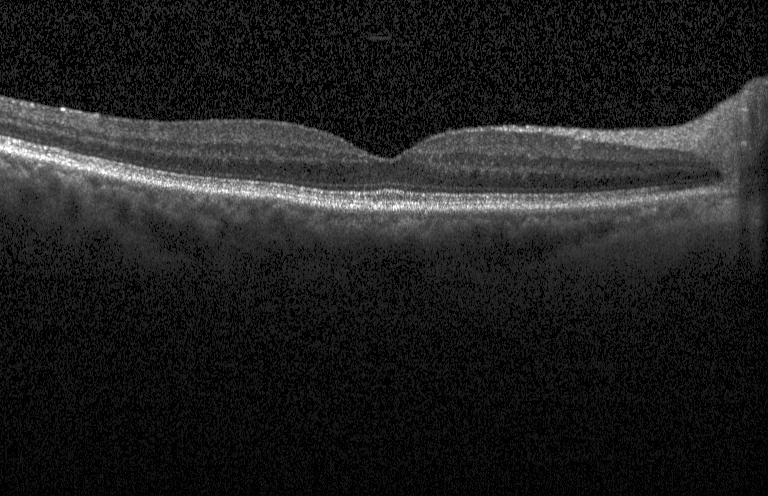

Finding: no CNV, no DME, and no drusen.